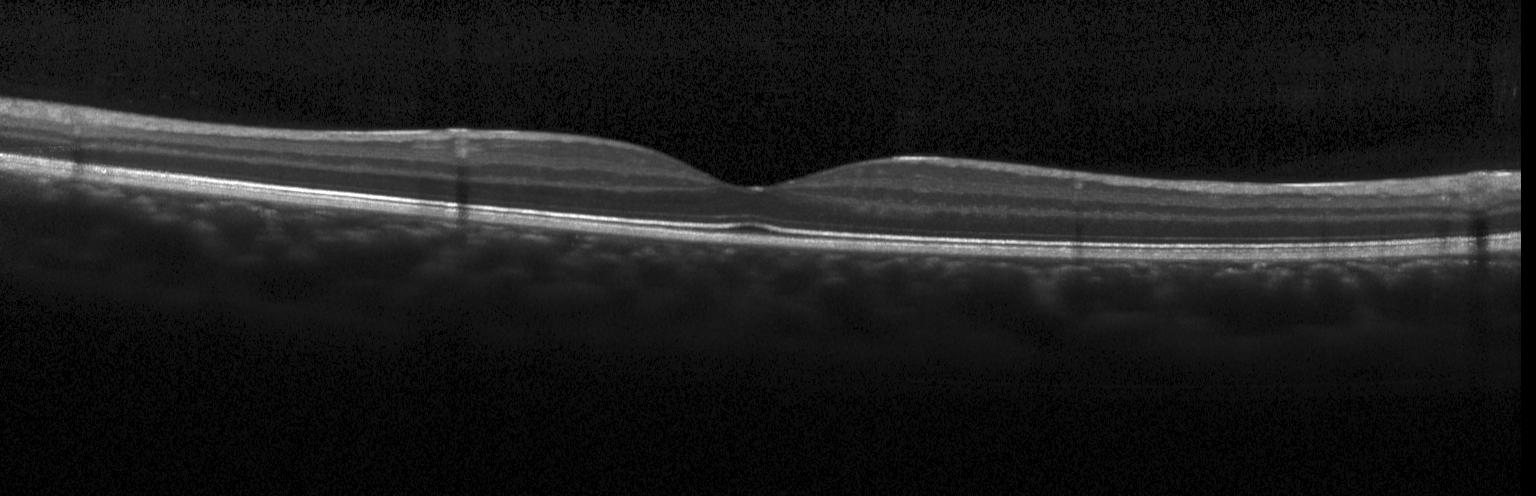 Centered on the fovea · acquired on a Heidelberg Spectralis · OCT B-scan.
Diagnosis: neither CNV, DME, nor drusen.